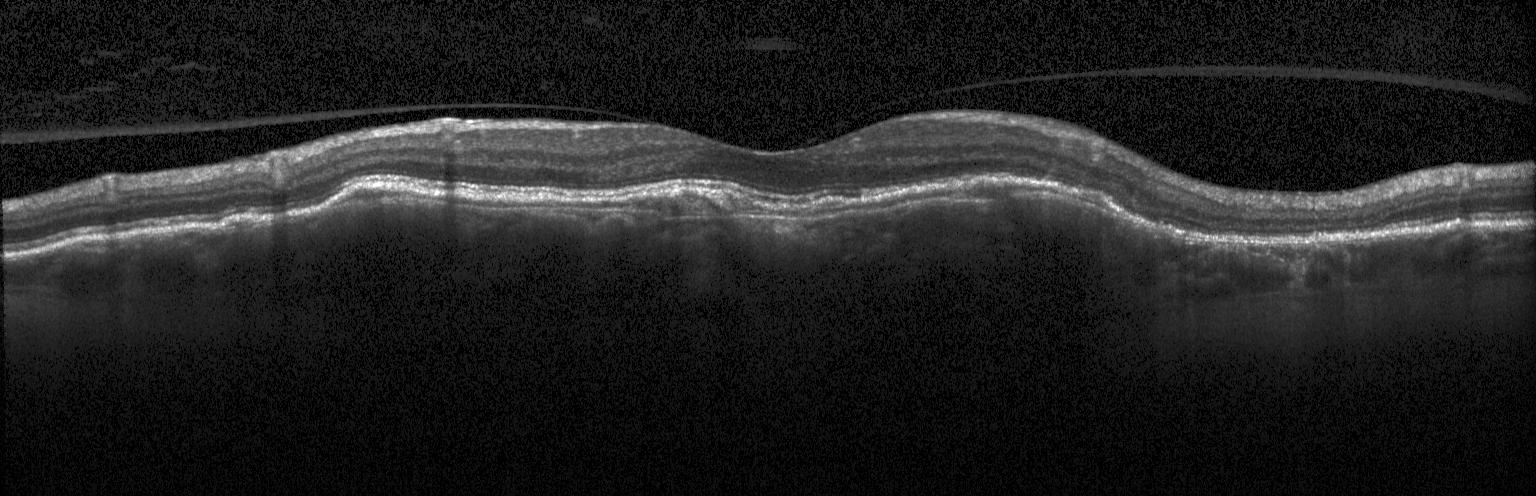
OCT B-scan; Heidelberg Spectralis; spectral-domain OCT.
CNV.